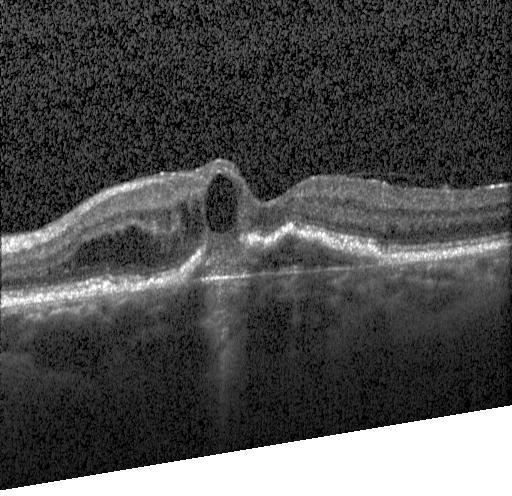
Optical coherence tomography scan; Heidelberg Spectralis — Impression: a choroidal neovascular membrane.